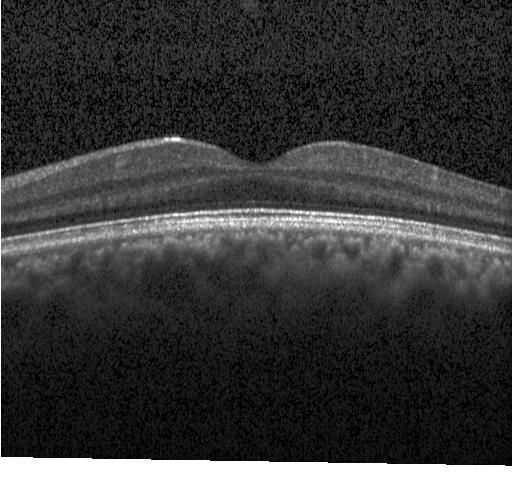
OCT B-scan.
Finding: no choroidal neovascularization, no diabetic macular edema, and no drusen.